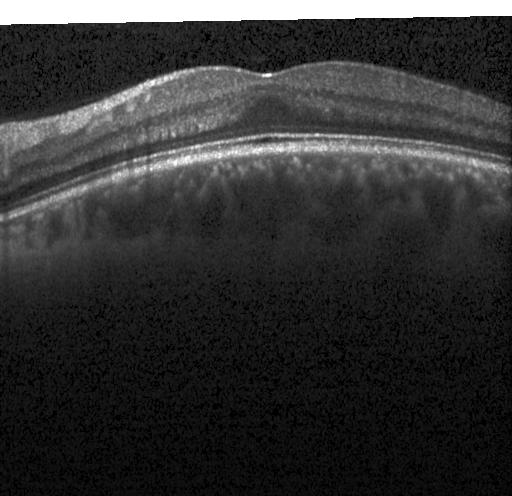 Optical coherence tomography scan — The scan shows neither choroidal neovascularization, diabetic macular edema, nor drusen.